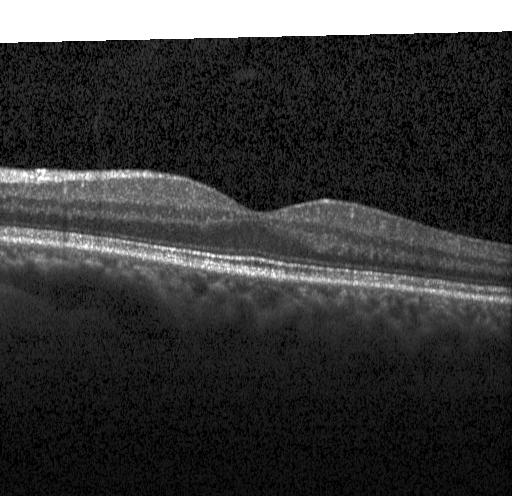
Acquired on a Heidelberg Spectralis · macular scan · OCT B-scan · spectral-domain optical coherence tomography — Macular OCT: no evidence of choroidal neovascularization, diabetic macular edema, or drusen.